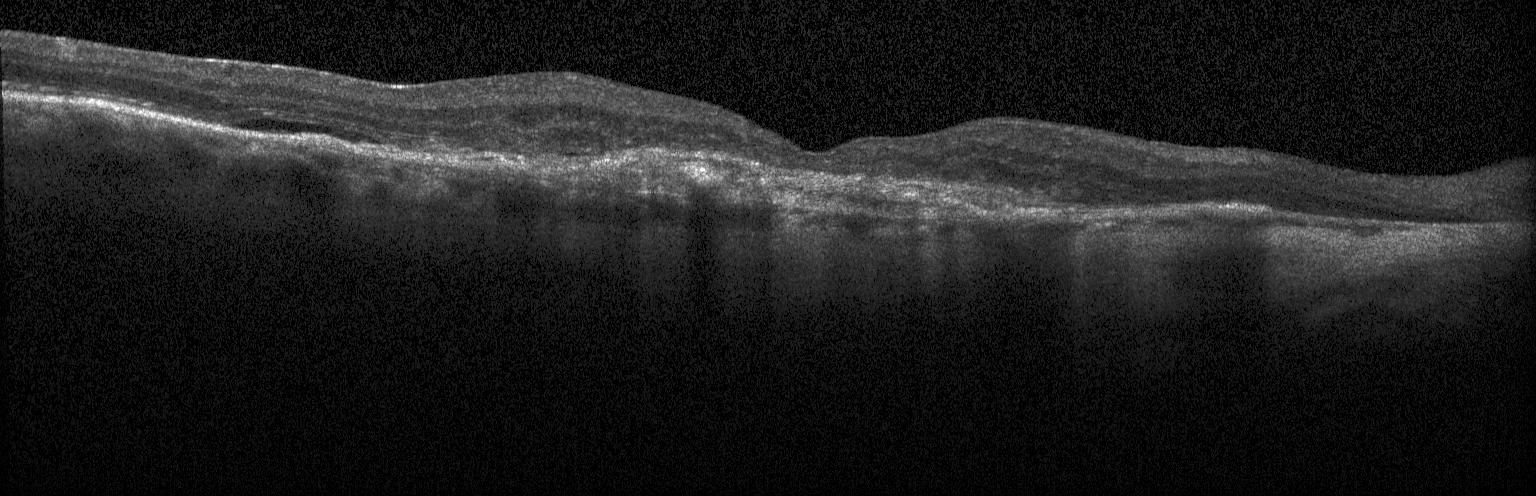
OCT B-scan showing choroidal neovascularization (CNV).